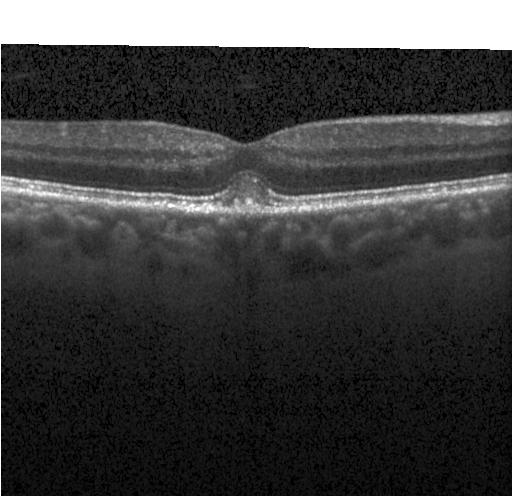 Spectral-domain OCT B-scan: drusen.